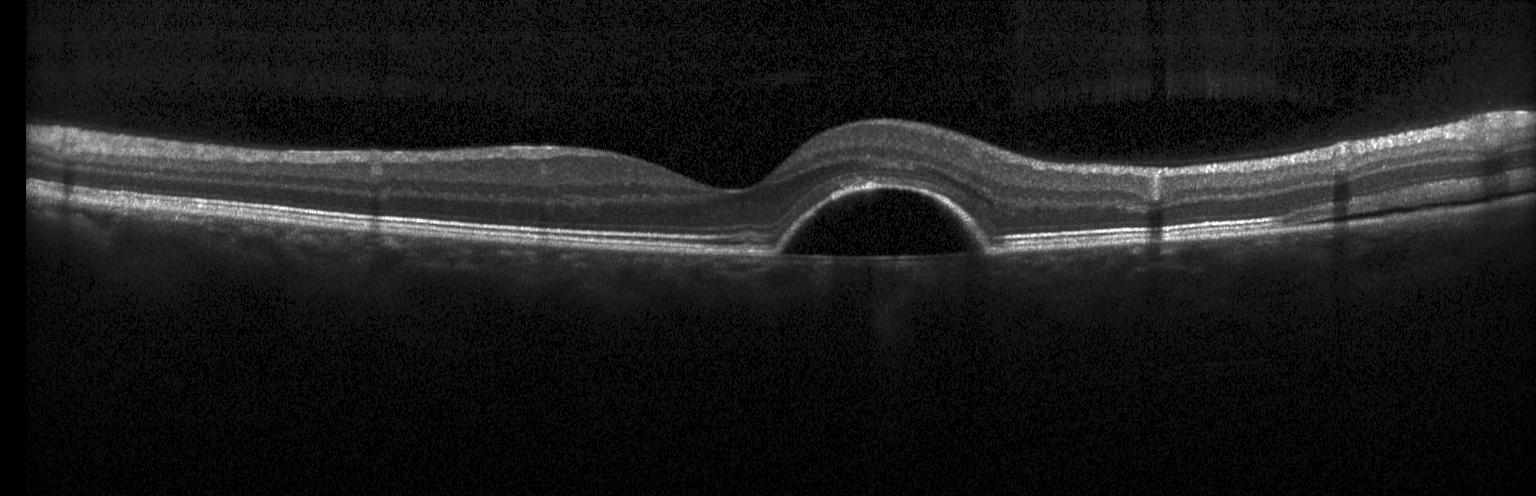
SD-OCT, centered on the fovea, Heidelberg Spectralis OCT system, retinal OCT B-scan
OCT finding: a choroidal neovascular membrane.